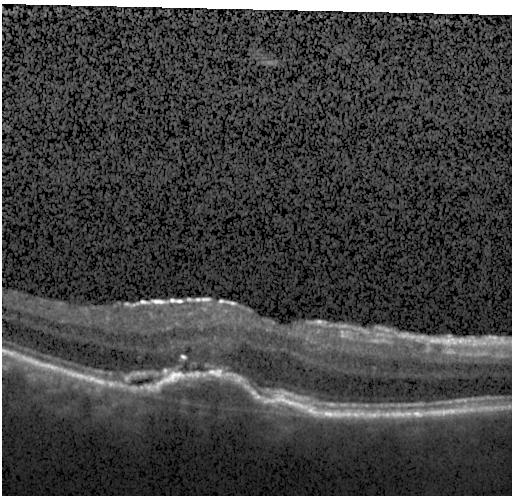
OCT B-scan, acquired on a Heidelberg Spectralis, macular scan, spectral-domain optical coherence tomography. Impression: a choroidal neovascular membrane.